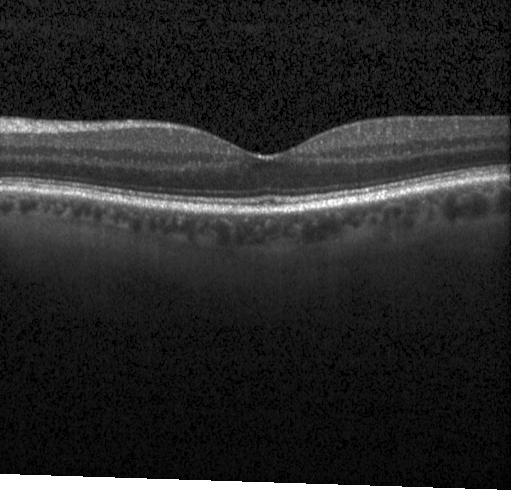

Dx: no choroidal neovascularization, diabetic macular edema, or drusen.